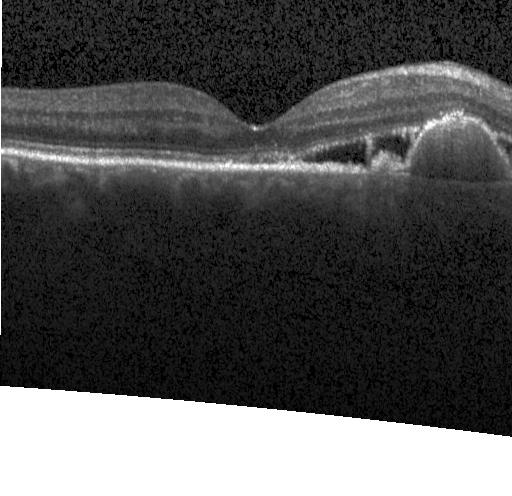

Assessment: CNV.